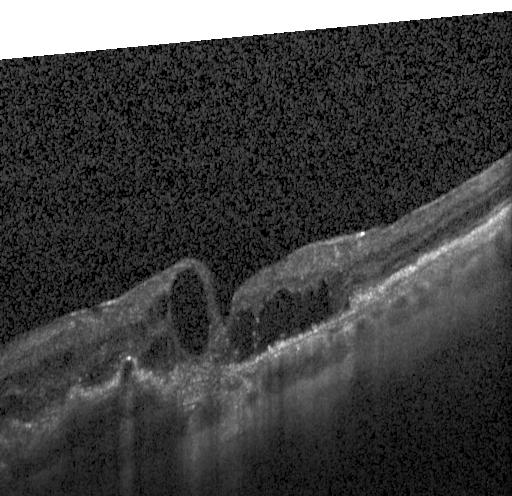

OCT line scan
Diagnosis: choroidal neovascularization.